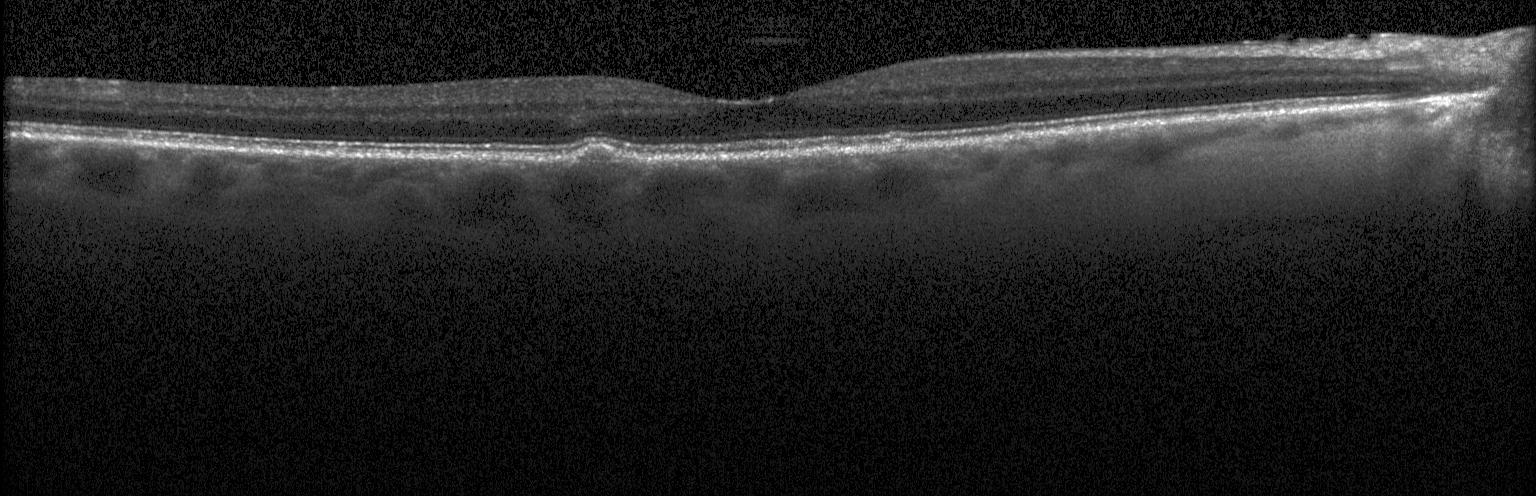

Retinal OCT cross-section. Centered on the fovea. Impression: multiple drusen.